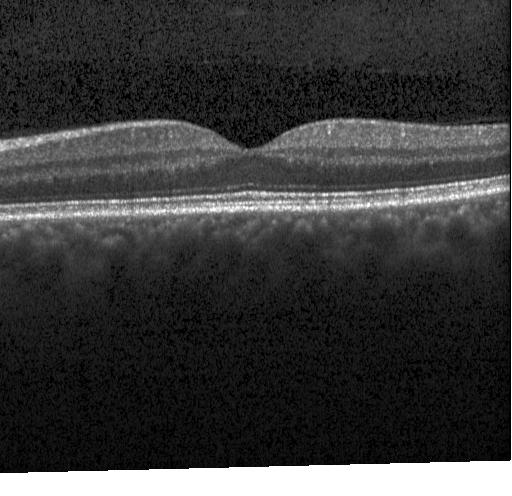 Through the macula, spectral-domain OCT, instrument: Heidelberg Spectralis, optical coherence tomography scan. Diagnosis: no choroidal neovascularization, no diabetic macular edema, and no drusen.